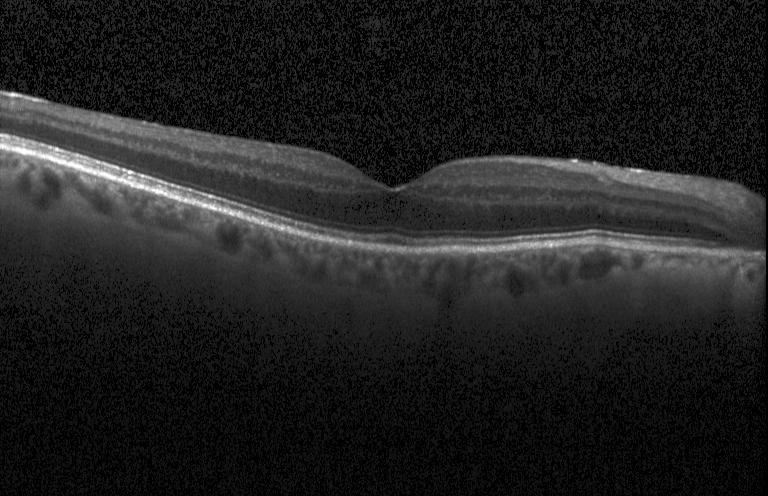

Acquired on a Heidelberg Spectralis. Horizontal scan through the fovea. Retinal OCT B-scan
Dx: neither CNV, DME, nor drusen.